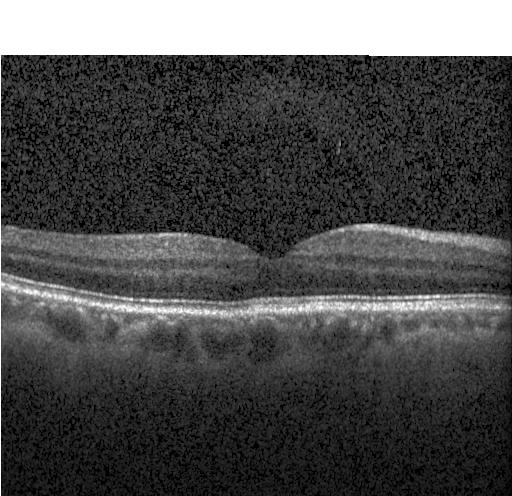

Dx: no choroidal neovascularization, no diabetic macular edema, and no drusen.